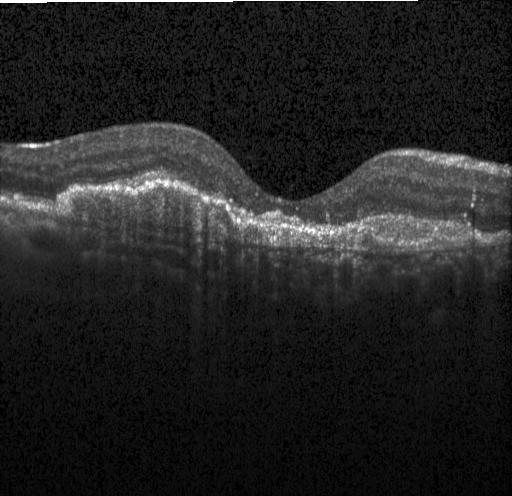
Diagnosis: CNV.